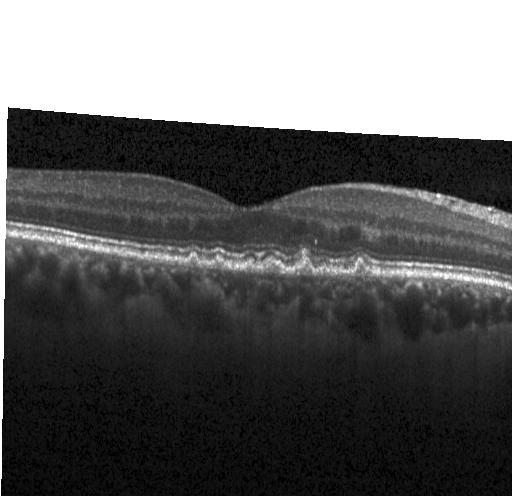 Centered on the fovea · spectral-domain OCT · OCT B-scan · Heidelberg Spectralis OCT system.
Dx: multiple drusen.